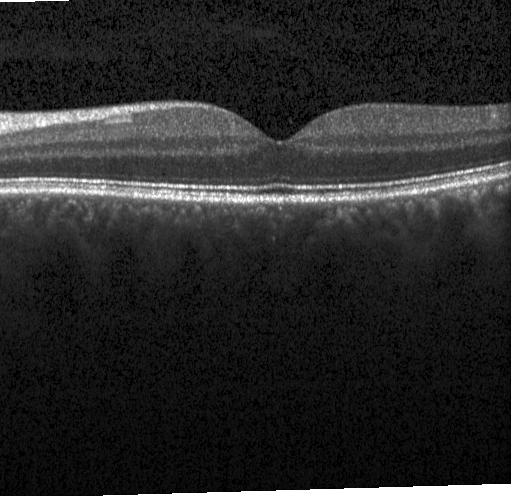

This B-scan demonstrates no choroidal neovascularization, no diabetic macular edema, and no drusen.